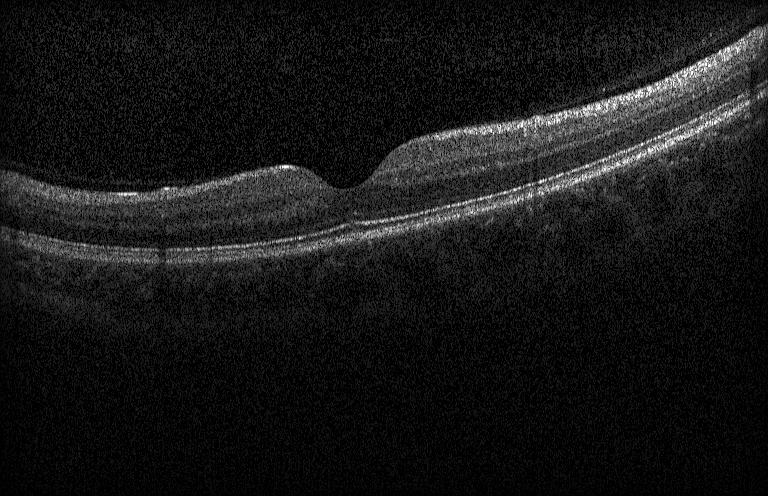

Retinal OCT B-scan · acquired on a Heidelberg Spectralis.
Finding: neither choroidal neovascularization, diabetic macular edema, nor drusen.